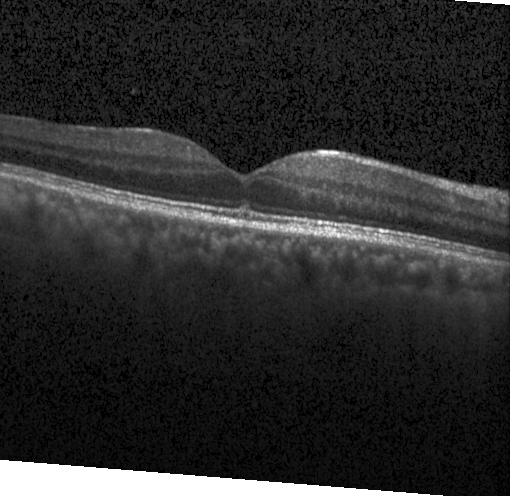

Macular OCT: no choroidal neovascularization, diabetic macular edema, or drusen.